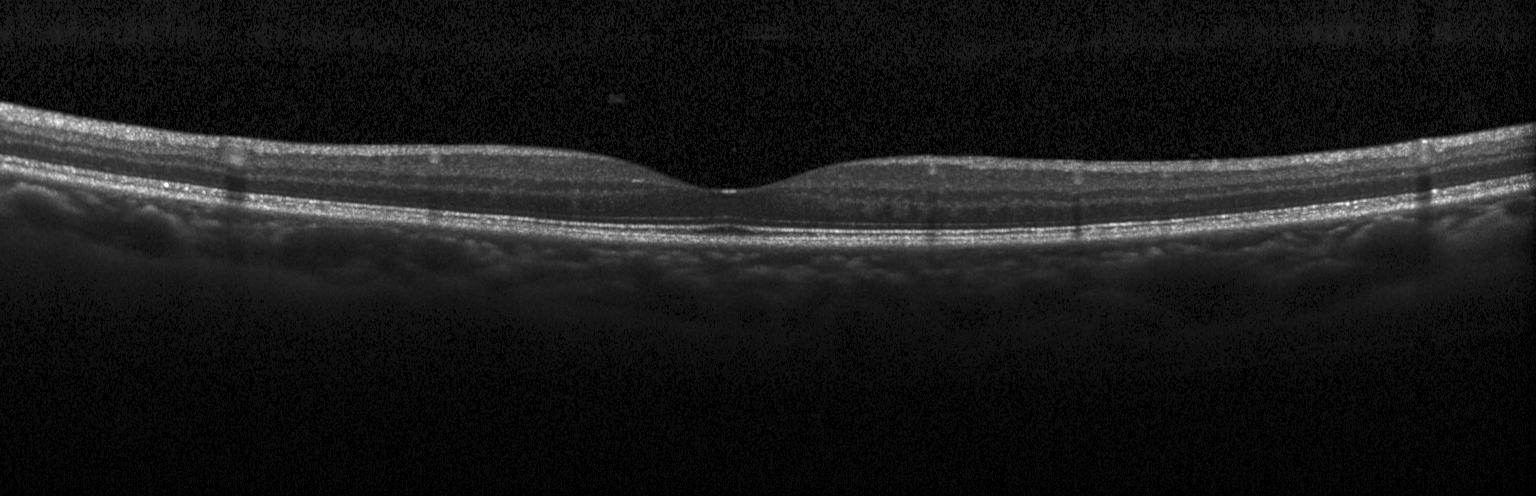

Retinal OCT B-scan, acquired on a Heidelberg Spectralis.
Macular OCT: no CNV, DME, or drusen.